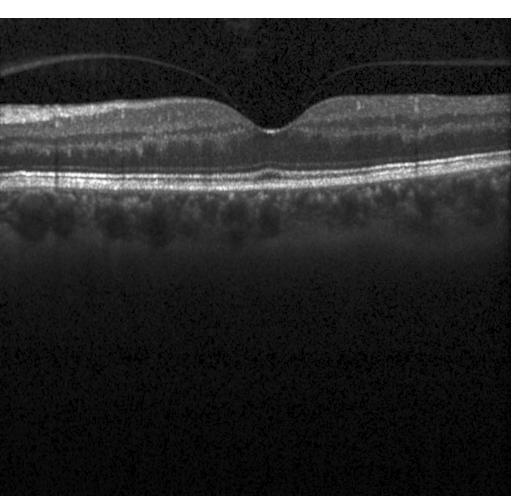

OCT scan showing neither choroidal neovascularization, diabetic macular edema, nor drusen.